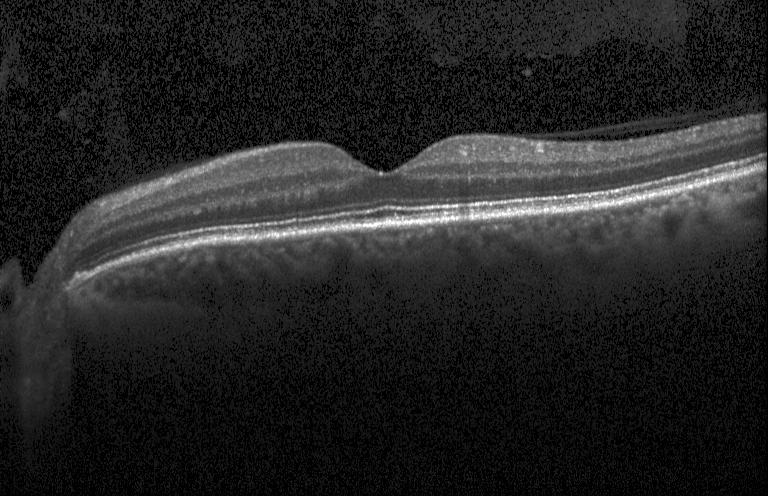

Spectral-domain OCT B-scan: no CNV, DME, or drusen.